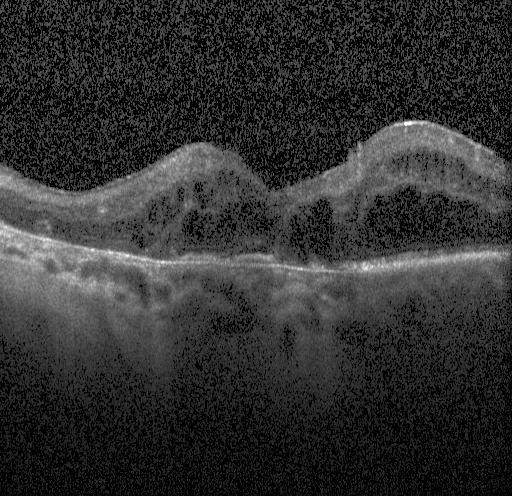 Retinal OCT cross-section showing choroidal neovascularization (CNV).